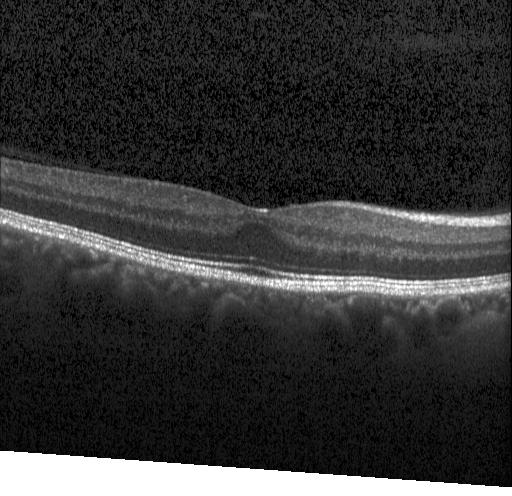 OCT scan showing no choroidal neovascularization, no diabetic macular edema, and no drusen.